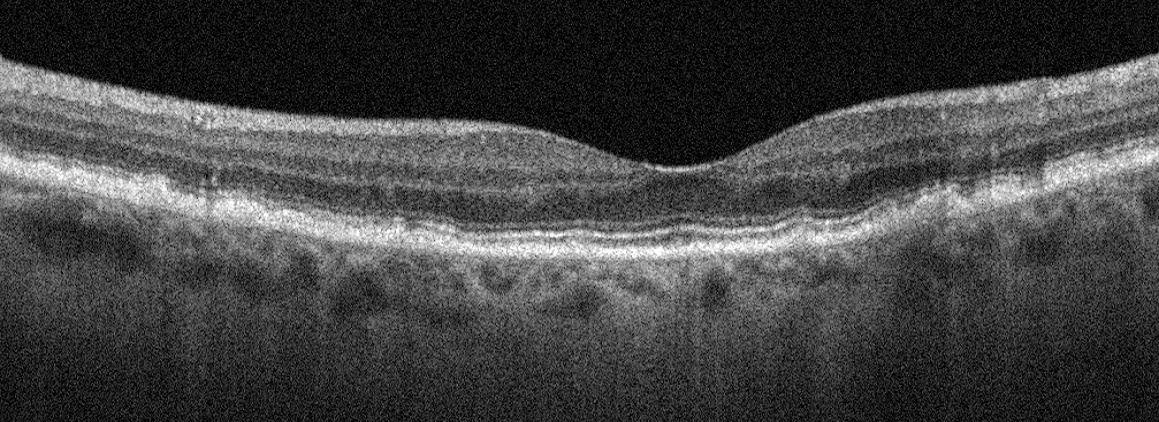 Left eye · OCT line scan. Age-related macular degeneration.